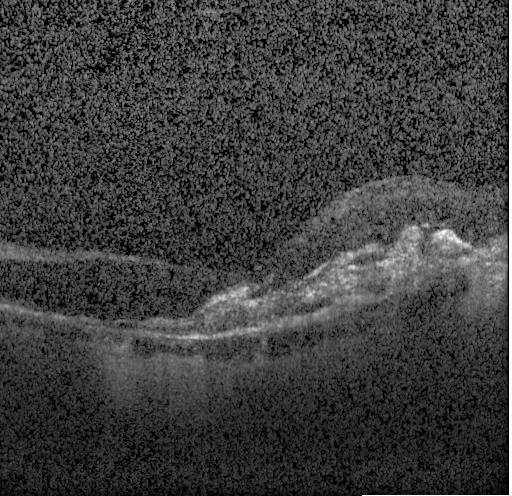 Macular OCT: a choroidal neovascular membrane.